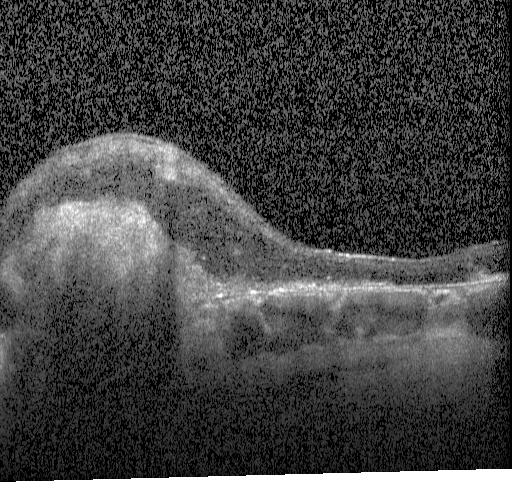

Instrument: Heidelberg Spectralis · OCT line scan · horizontal scan through the fovea · spectral-domain optical coherence tomography — Diagnosis: a choroidal neovascular membrane.